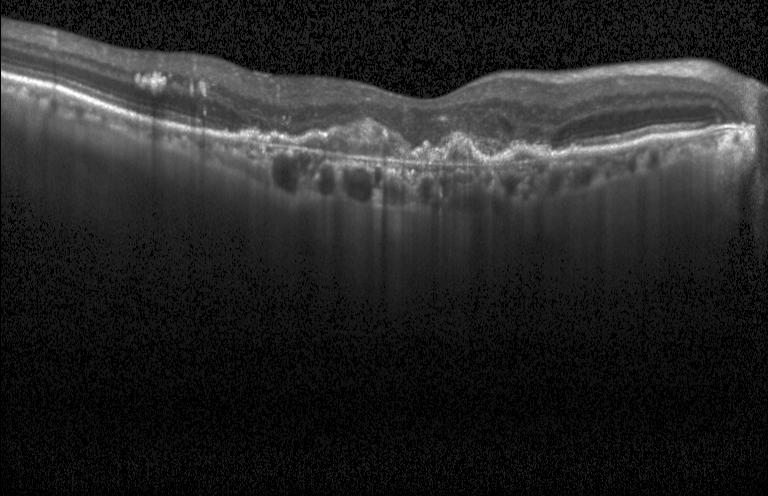

Impression: a choroidal neovascular membrane.